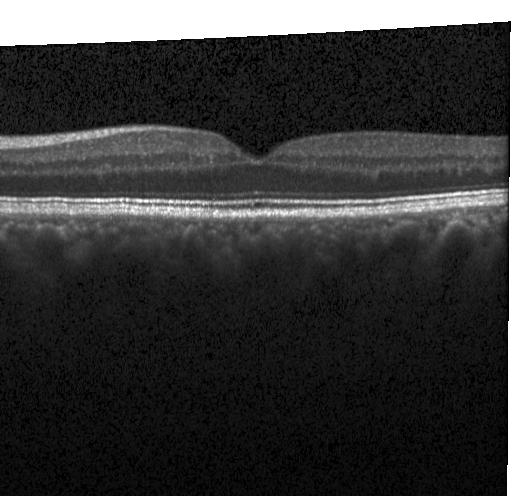

Heidelberg Spectralis, spectral-domain optical coherence tomography, horizontal scan through the fovea, optical coherence tomography scan. This B-scan demonstrates no evidence of choroidal neovascularization, diabetic macular edema, or drusen.